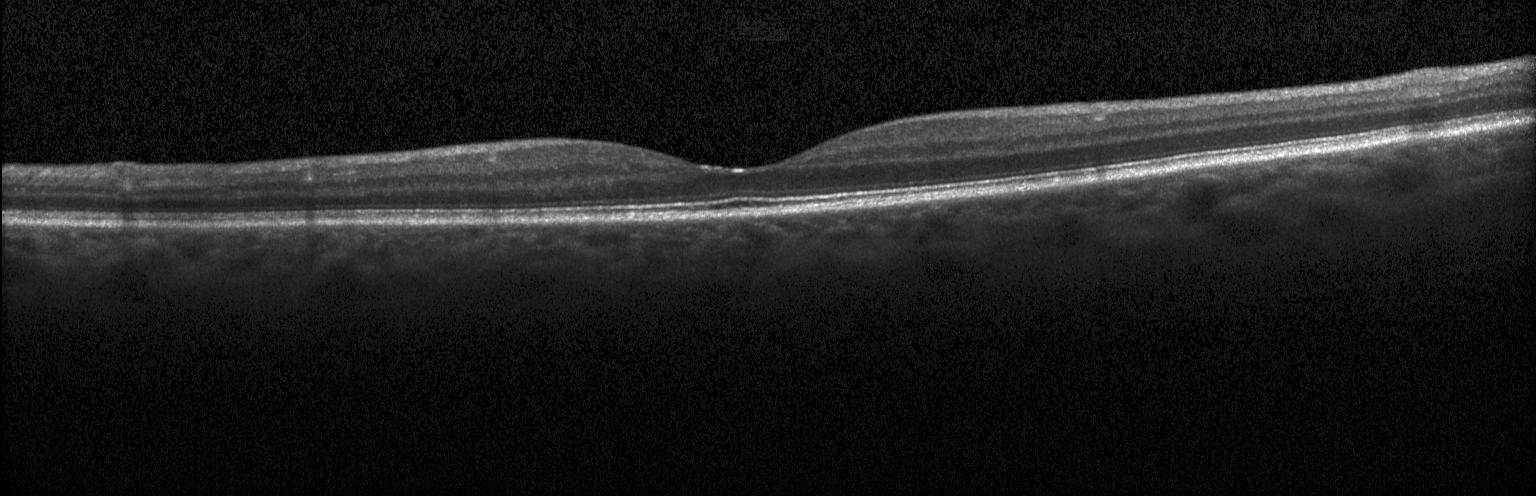
OCT B-scan, spectral-domain OCT, fovea-centered, instrument: Heidelberg Spectralis
Diagnosis: neither choroidal neovascularization, diabetic macular edema, nor drusen.